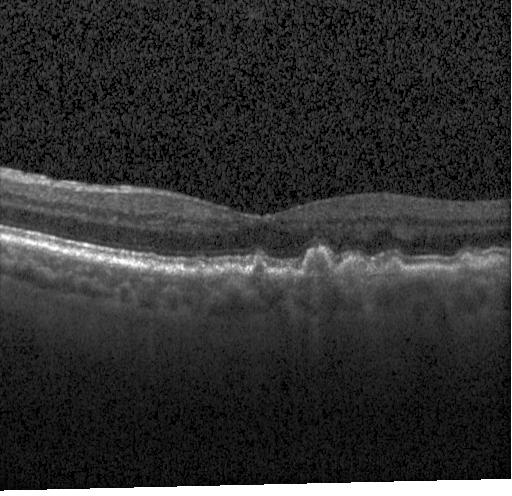 Optical coherence tomography scan; acquired on a Heidelberg Spectralis
The scan shows sub-RPE drusenoid deposits.